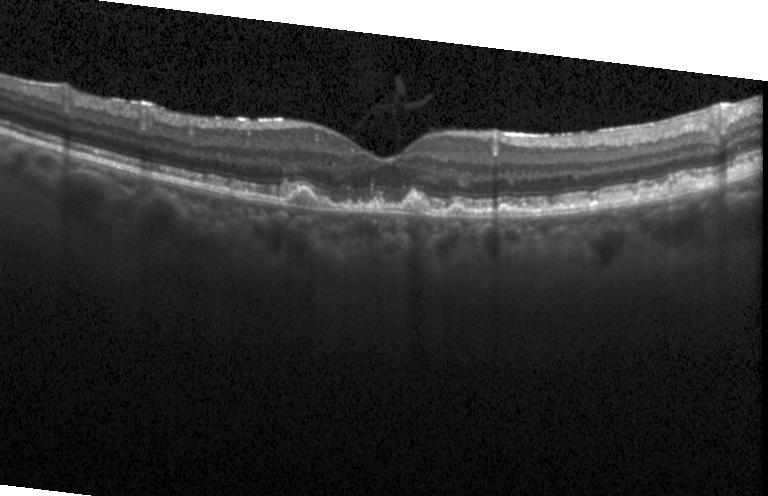
Dx: sub-RPE drusenoid deposits.